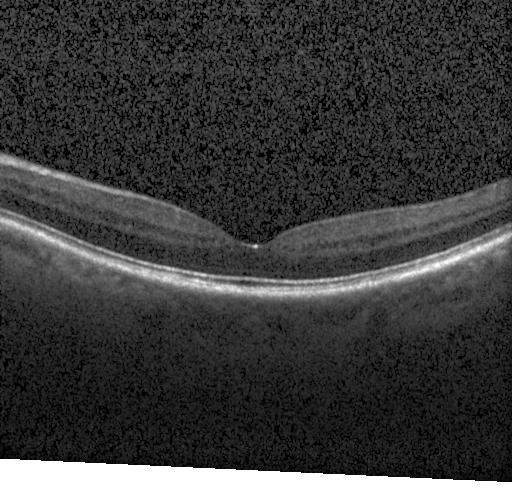 Through the macula · acquired on a Heidelberg Spectralis · optical coherence tomography B-scan.
This B-scan demonstrates neither choroidal neovascularization, diabetic macular edema, nor drusen.